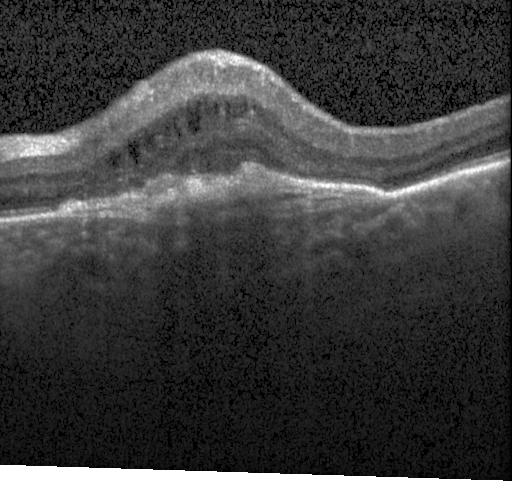
Through the macula; OCT B-scan — Choroidal neovascularization.